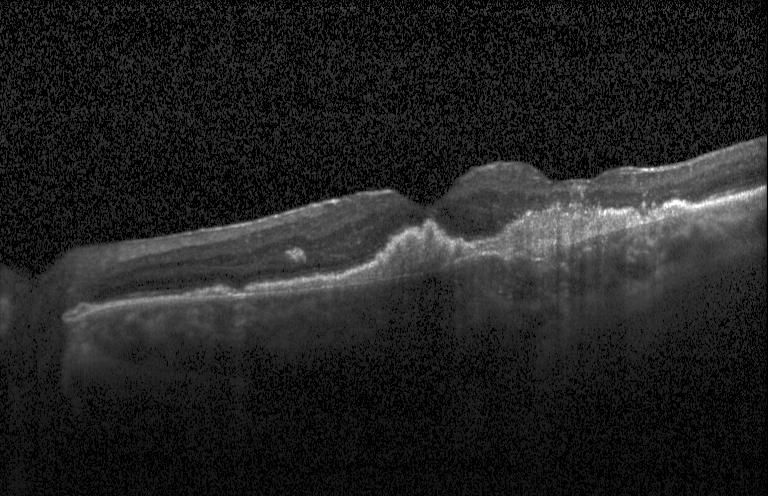

Retinal OCT cross-section.
Assessment: a choroidal neovascular membrane.